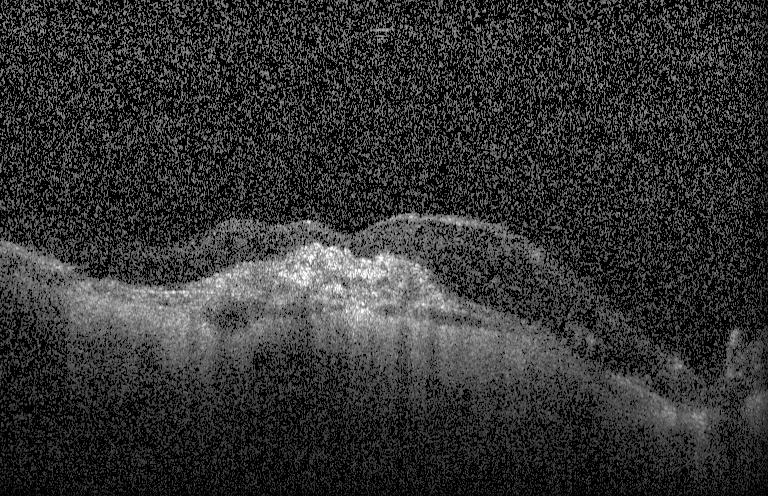 Dx: a choroidal neovascular membrane.